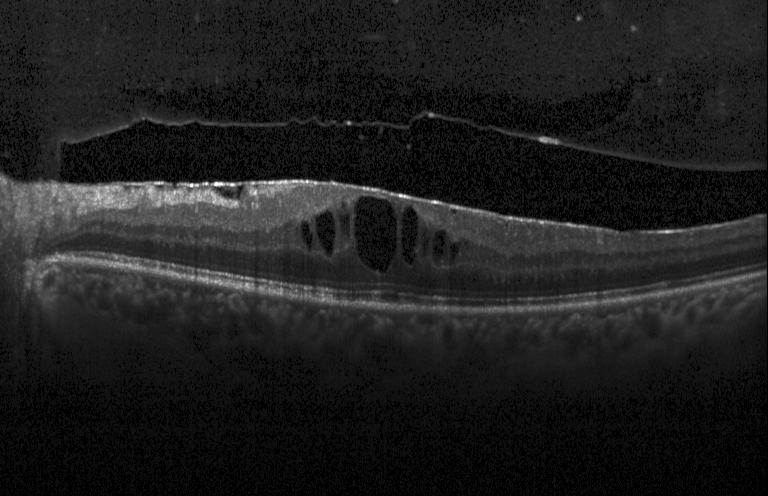

Impression: DME.